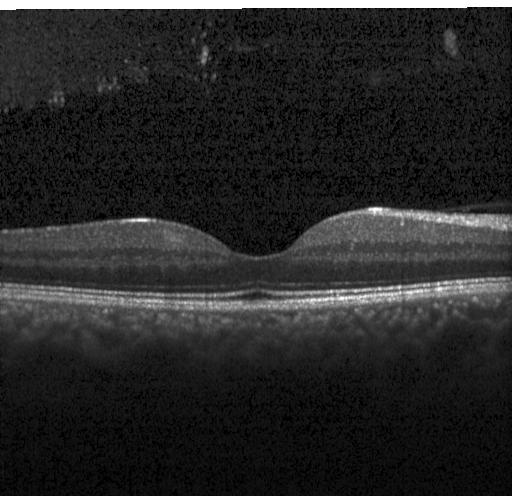
Optical coherence tomography scan
Finding: no choroidal neovascularization, diabetic macular edema, or drusen.